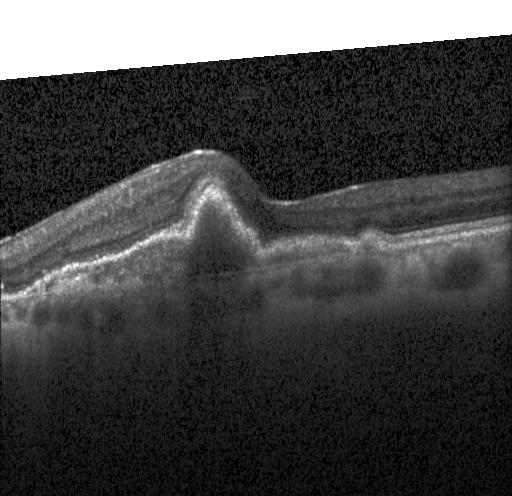
SD-OCT. Heidelberg Spectralis. Fovea-centered. Optical coherence tomography B-scan — Finding: a choroidal neovascular membrane.